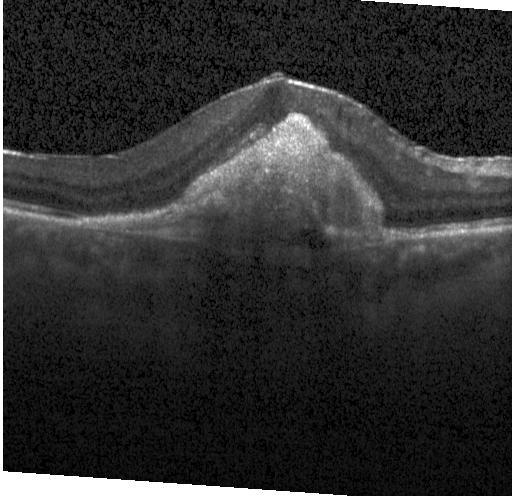
Optical coherence tomography B-scan. Macular scan. Assessment: choroidal neovascularization (CNV).